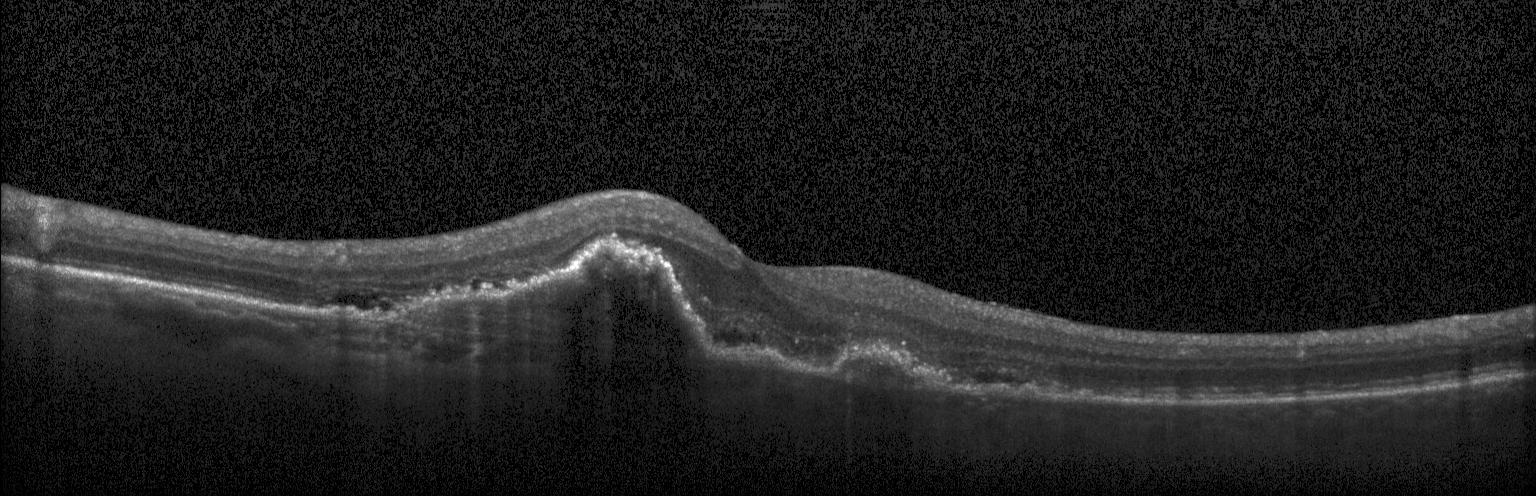

OCT B-scan — The scan shows CNV.